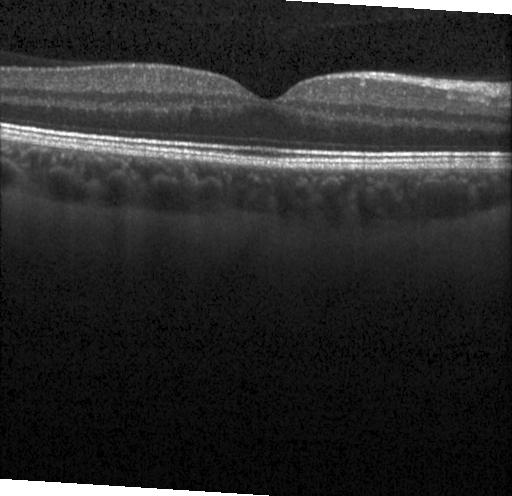 The scan shows neither CNV, DME, nor drusen.